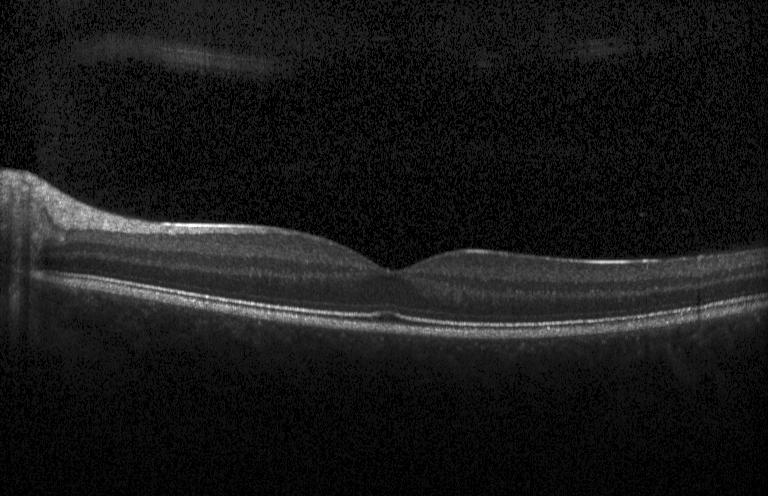 Retinal OCT cross-section · instrument: Heidelberg Spectralis. Finding: no evidence of choroidal neovascularization, diabetic macular edema, or drusen.